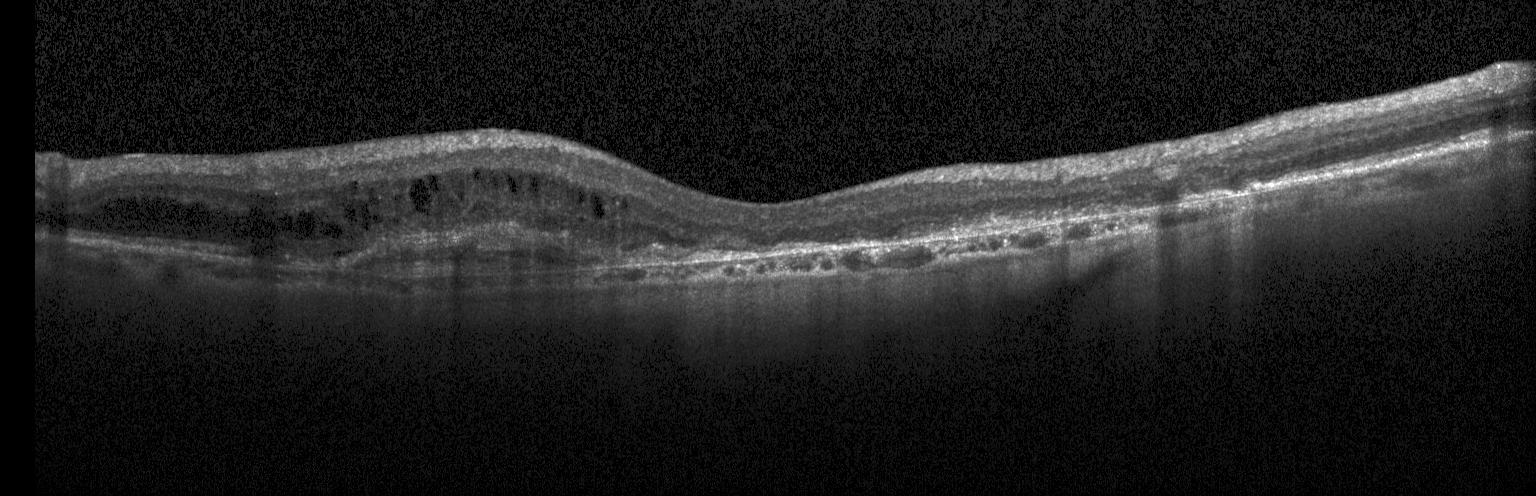
Fovea-centered. Optical coherence tomography B-scan
Finding: a choroidal neovascular membrane.